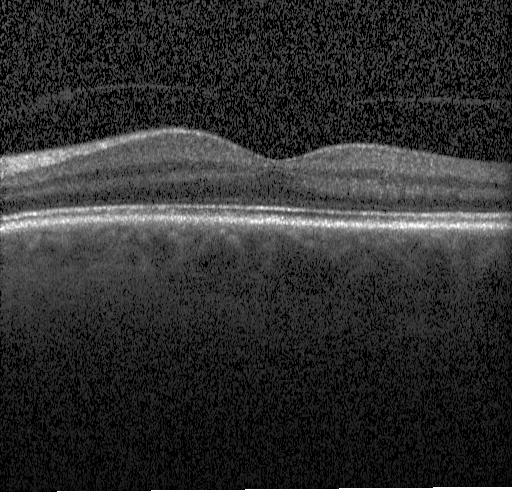
Acquired on a Heidelberg Spectralis · optical coherence tomography B-scan. Diagnosis: no evidence of choroidal neovascularization, diabetic macular edema, or drusen.